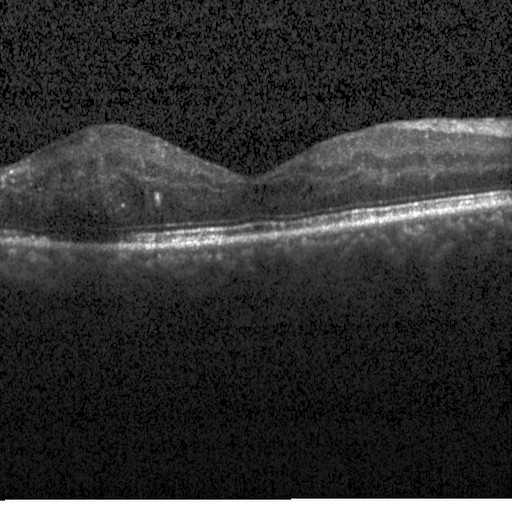
OCT B-scan showing diabetic macular edema (DME).